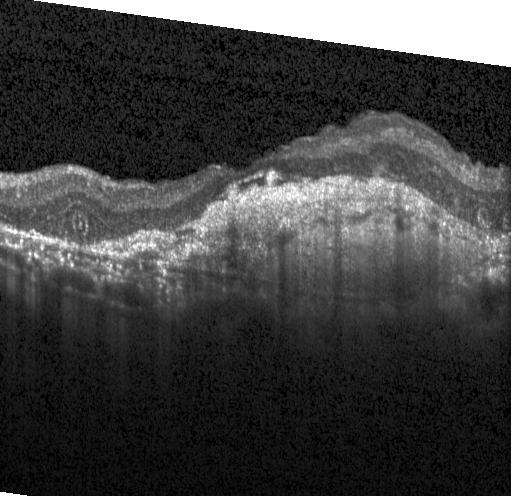

Finding: a choroidal neovascular membrane.